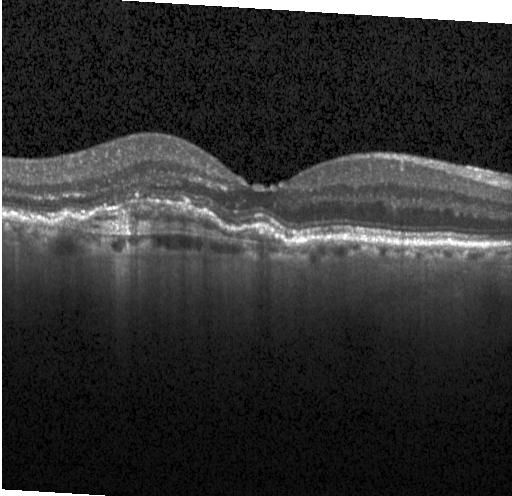 Optical coherence tomography B-scan · Heidelberg Spectralis OCT system · macular scan.
Diagnosis: choroidal neovascularization.